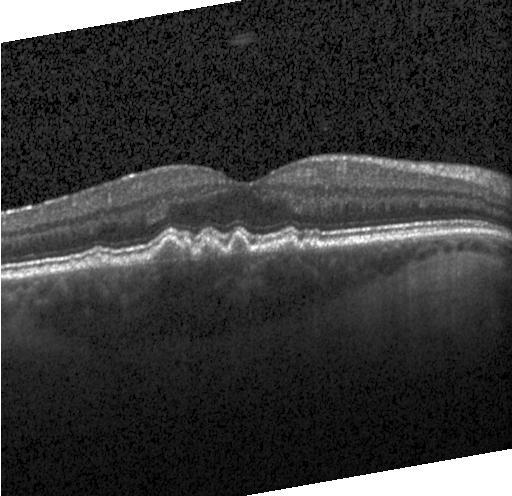

Heidelberg Spectralis, macular scan, spectral-domain OCT, OCT B-scan
The scan shows sub-RPE drusenoid deposits.